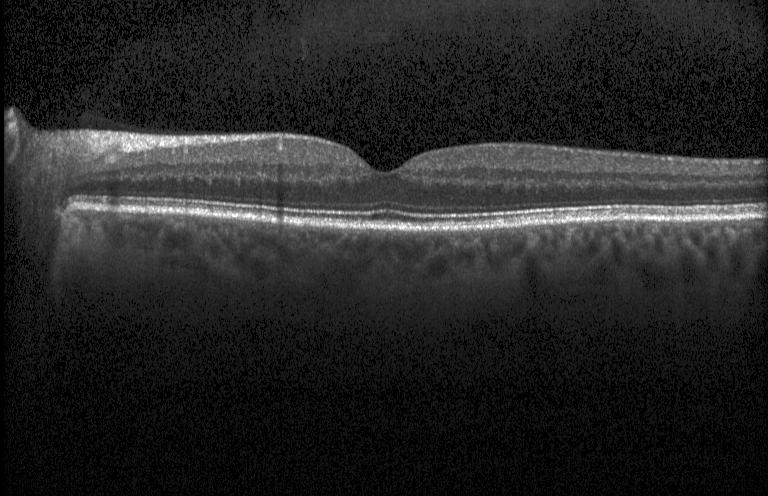

OCT B-scan. Dx: no evidence of CNV, DME, or drusen.